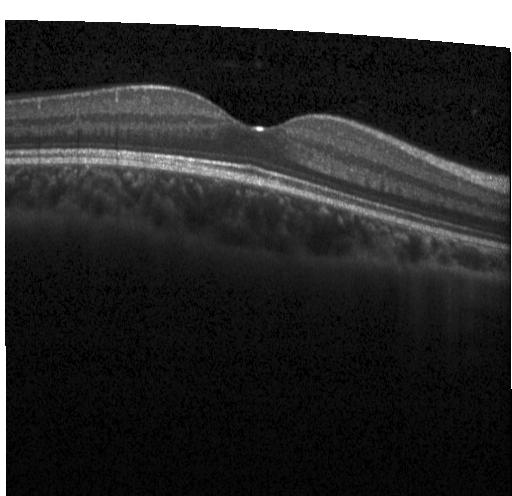
Fovea-centered. OCT line scan. Heidelberg Spectralis.
No choroidal neovascularization, diabetic macular edema, or drusen.